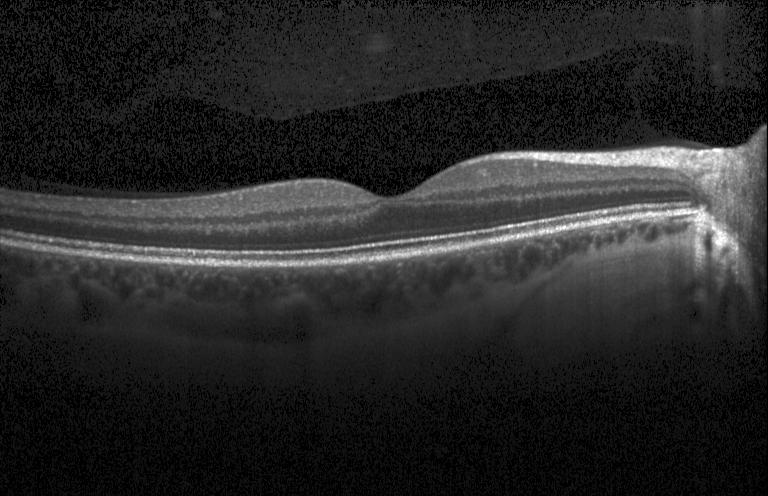 Retinal OCT B-scan, spectral-domain OCT.
OCT finding: no choroidal neovascularization, diabetic macular edema, or drusen.